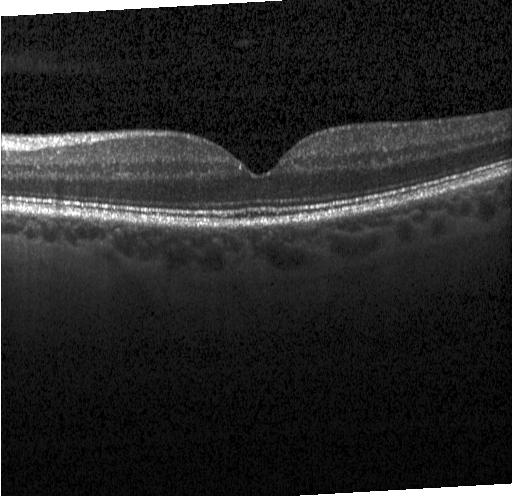
Spectral-domain OCT B-scan: no evidence of choroidal neovascularization, diabetic macular edema, or drusen.